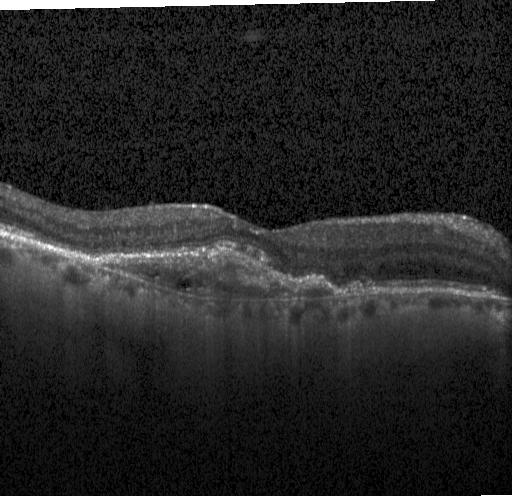 Diagnosis: a choroidal neovascular membrane.